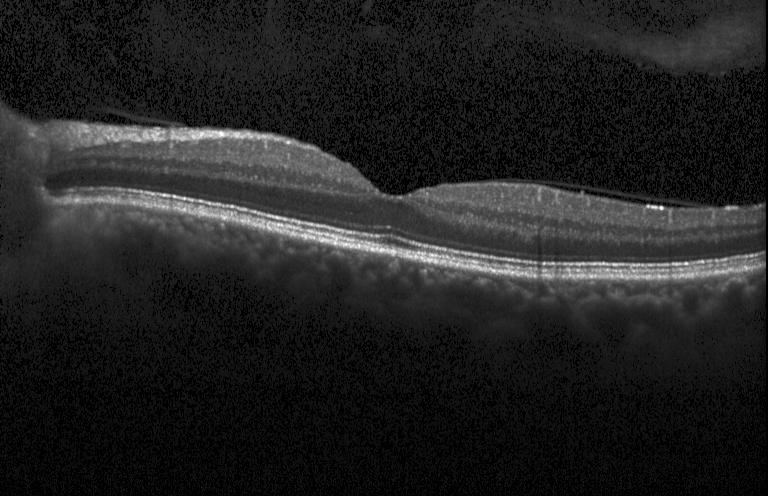 Retinal OCT cross-section.
Assessment: no choroidal neovascularization, diabetic macular edema, or drusen.